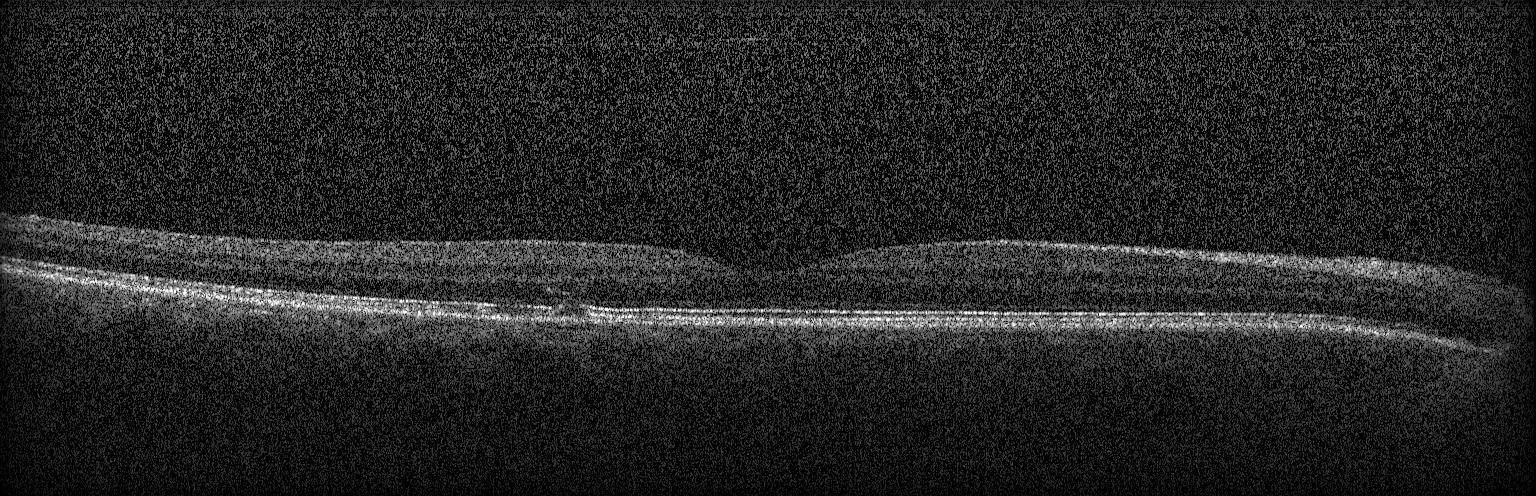 OCT line scan — Impression: neither choroidal neovascularization, diabetic macular edema, nor drusen.